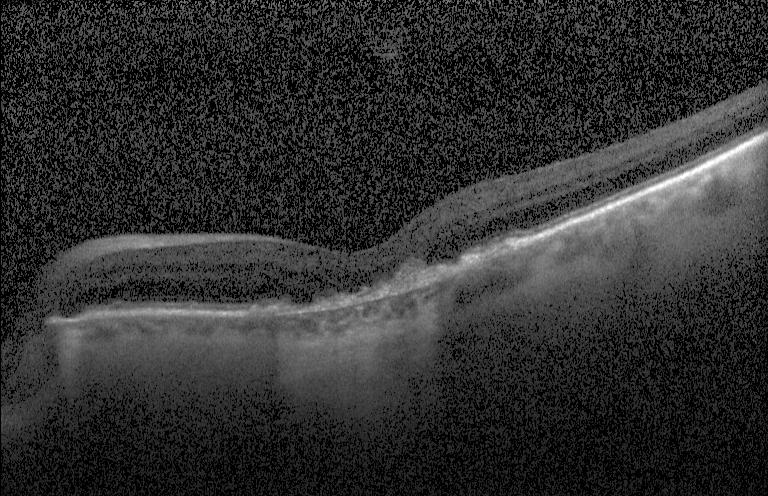 Optical coherence tomography scan; spectral-domain OCT.
This B-scan demonstrates CNV.